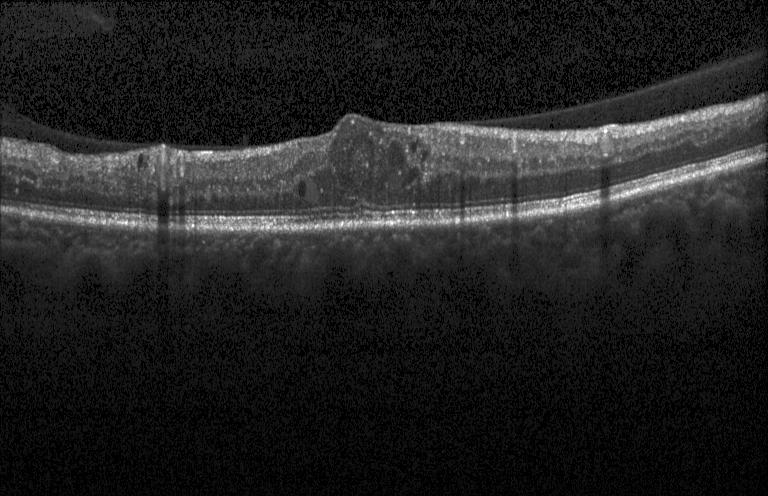 Spectral-domain OCT; centered on the fovea; Heidelberg Spectralis; optical coherence tomography B-scan
OCT finding: diabetic macular edema (DME).